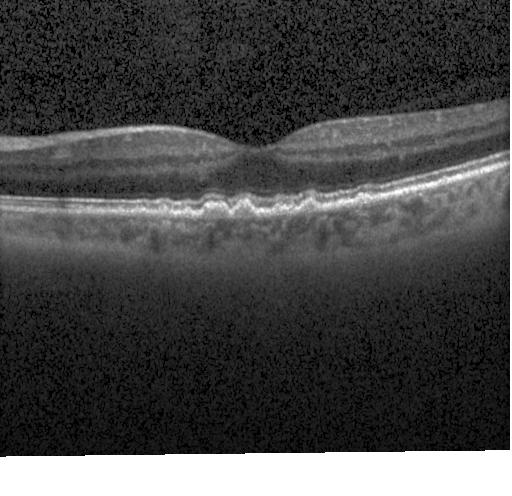

Retinal OCT B-scan, spectral-domain OCT — Diagnosis: drusen.